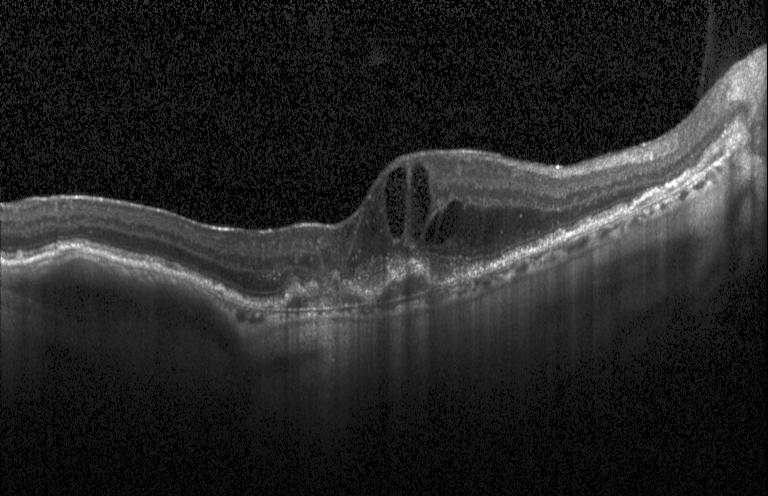

Choroidal neovascularization.